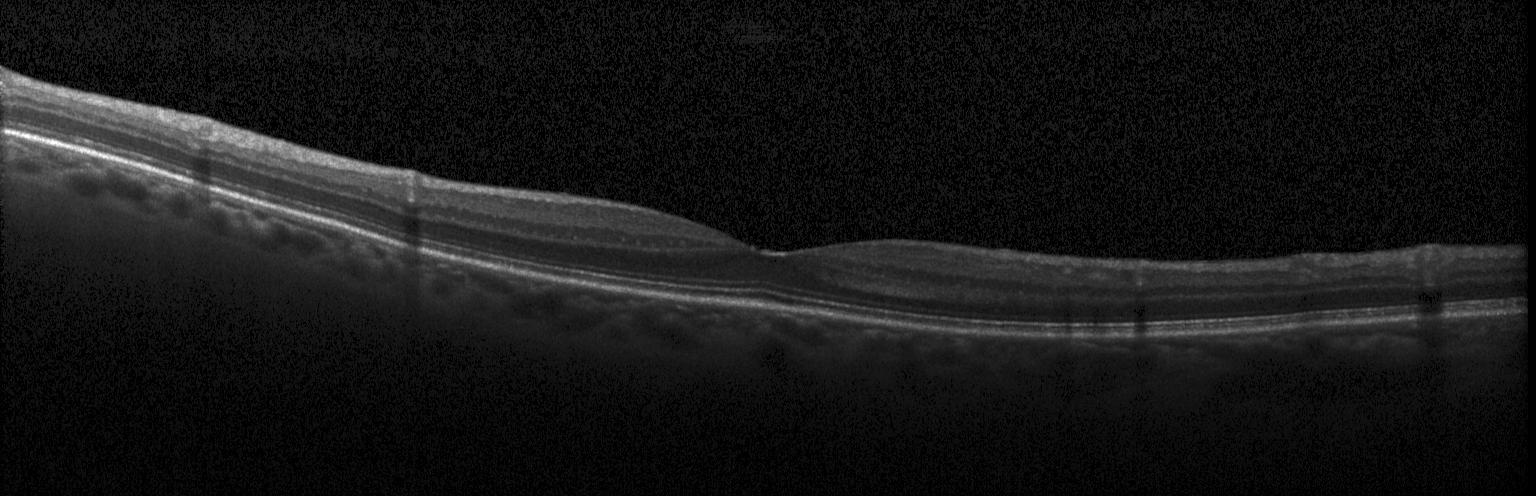
Through the macula; Heidelberg Spectralis; optical coherence tomography B-scan
Neither choroidal neovascularization, diabetic macular edema, nor drusen.